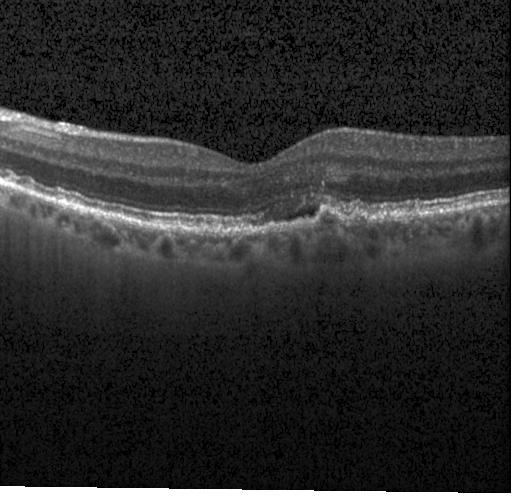 Dx: choroidal neovascularization (CNV).